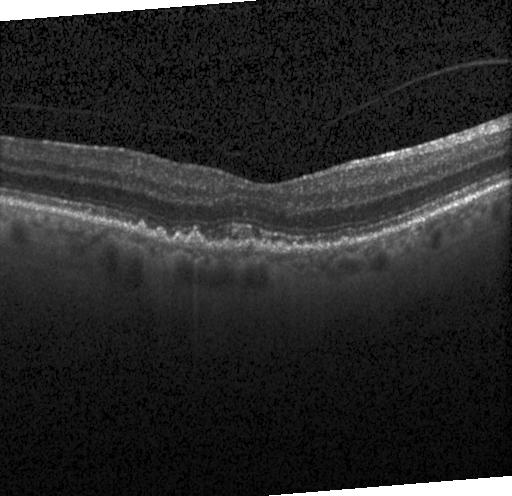

Diagnosis: sub-RPE drusenoid deposits.